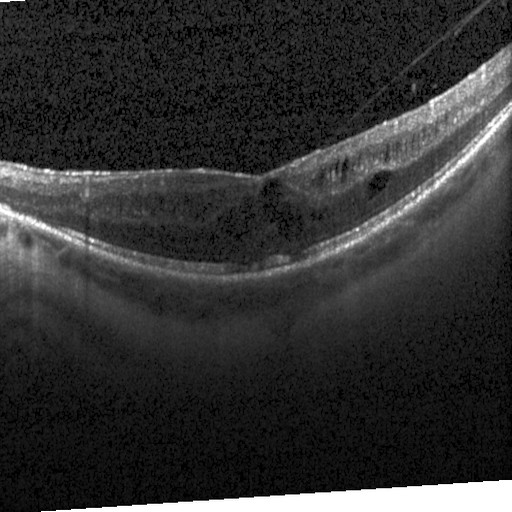 OCT finding: diabetic macular edema (DME).